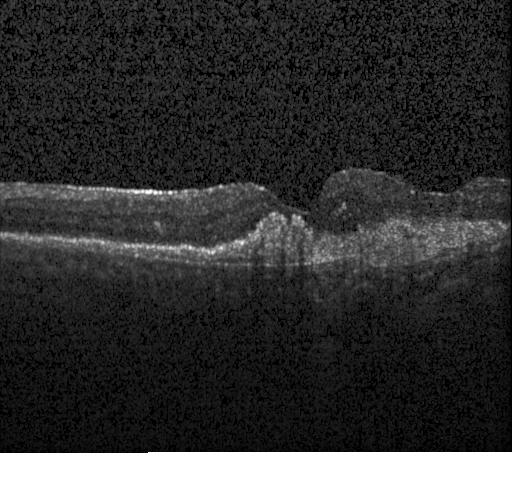 Retinal OCT B-scan, spectral-domain OCT. Assessment: a choroidal neovascular membrane.